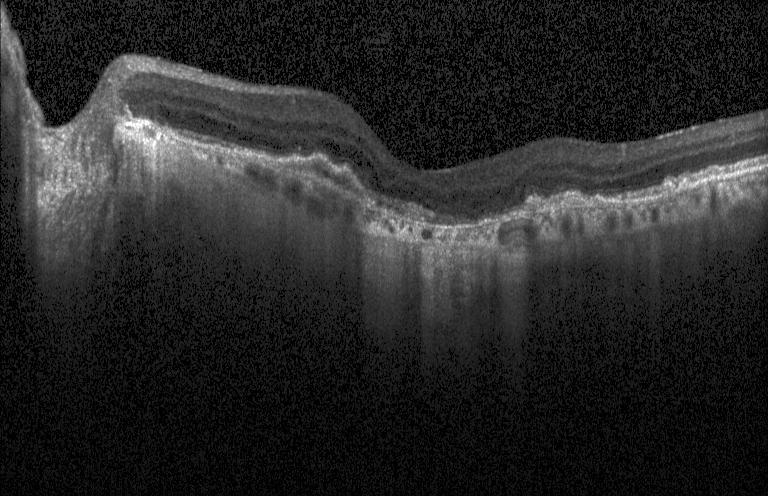 Acquired on a Heidelberg Spectralis, OCT line scan, spectral-domain optical coherence tomography
Impression: choroidal neovascularization.